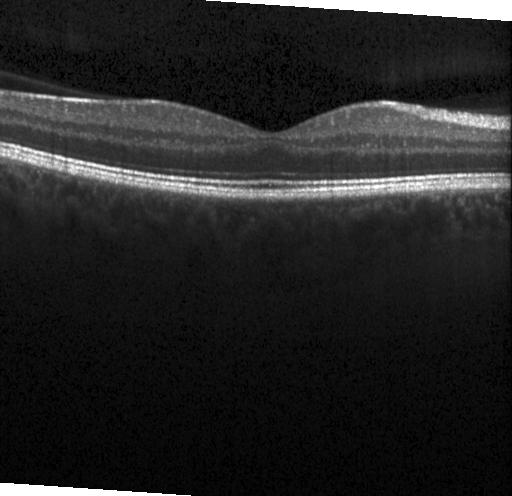

Instrument: Heidelberg Spectralis; fovea-centered; spectral-domain optical coherence tomography; optical coherence tomography B-scan.
No evidence of choroidal neovascularization, diabetic macular edema, or drusen.